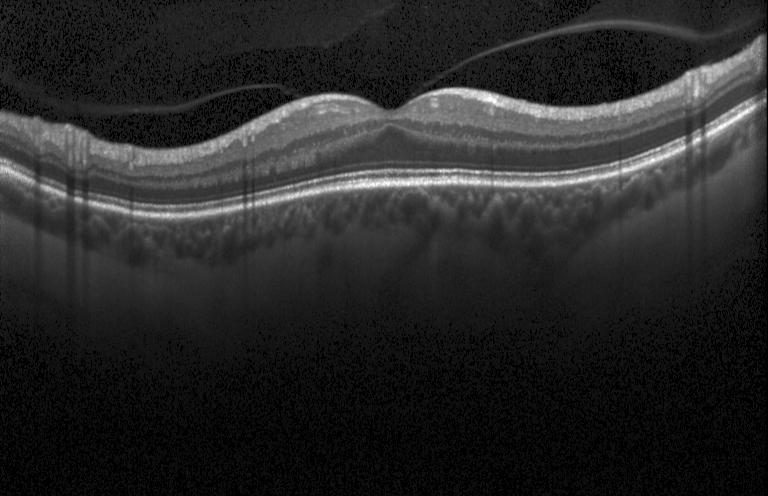

OCT scan showing neither choroidal neovascularization, diabetic macular edema, nor drusen.